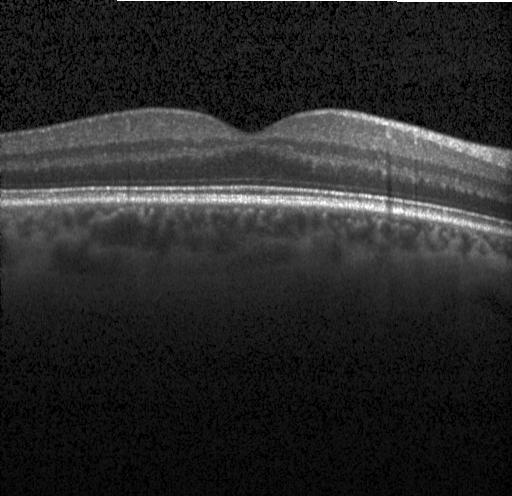 The scan shows no evidence of choroidal neovascularization, diabetic macular edema, or drusen.